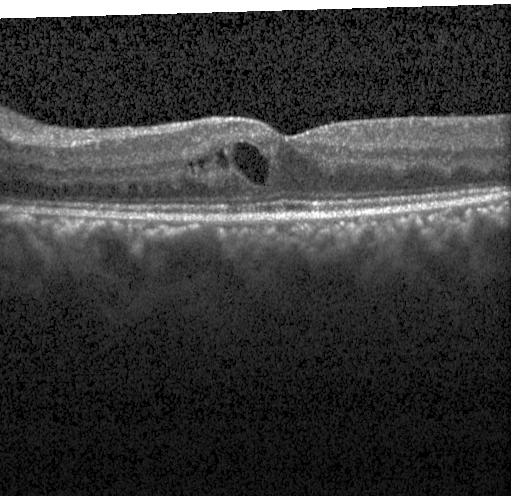
Impression: DME.